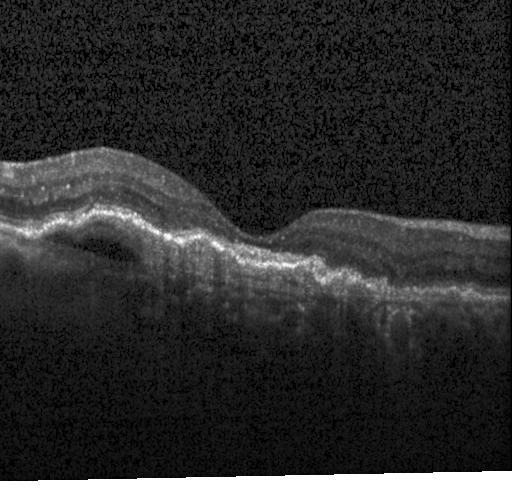
Optical coherence tomography scan
Diagnosis: CNV.